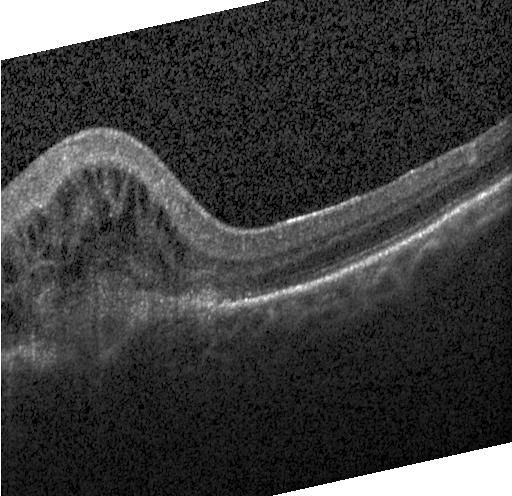
Spectral-domain OCT B-scan: choroidal neovascularization.